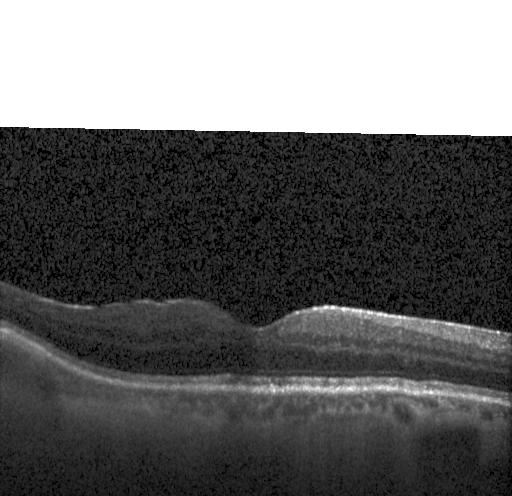
Optical coherence tomography B-scan — Finding: no CNV, no DME, and no drusen.